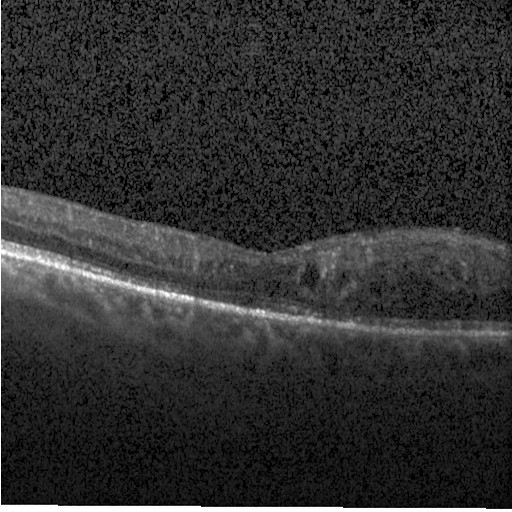 The scan shows diabetic macular edema (DME).